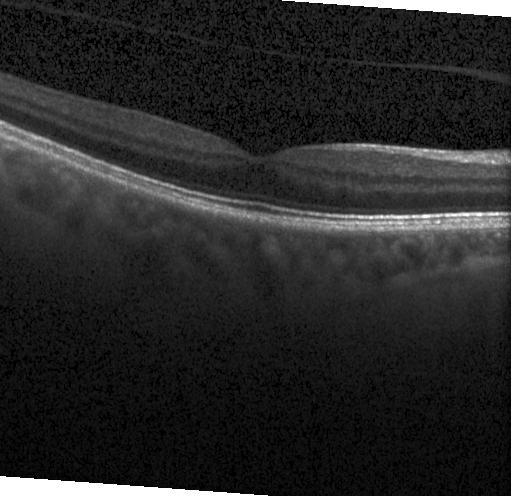
Heidelberg Spectralis, horizontal scan through the fovea, optical coherence tomography B-scan, spectral-domain OCT — This B-scan demonstrates no choroidal neovascularization, diabetic macular edema, or drusen.